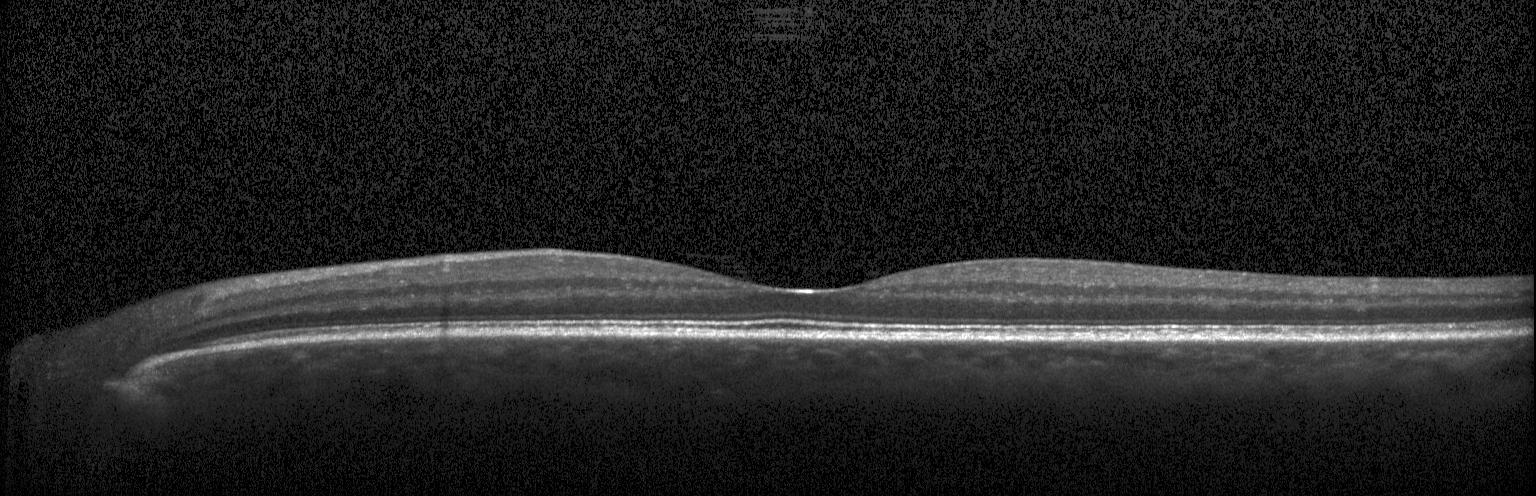

Impression: no choroidal neovascularization, no diabetic macular edema, and no drusen.